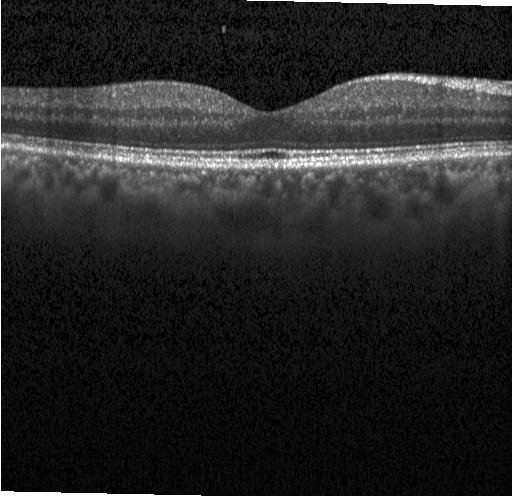

The scan shows neither choroidal neovascularization, diabetic macular edema, nor drusen.